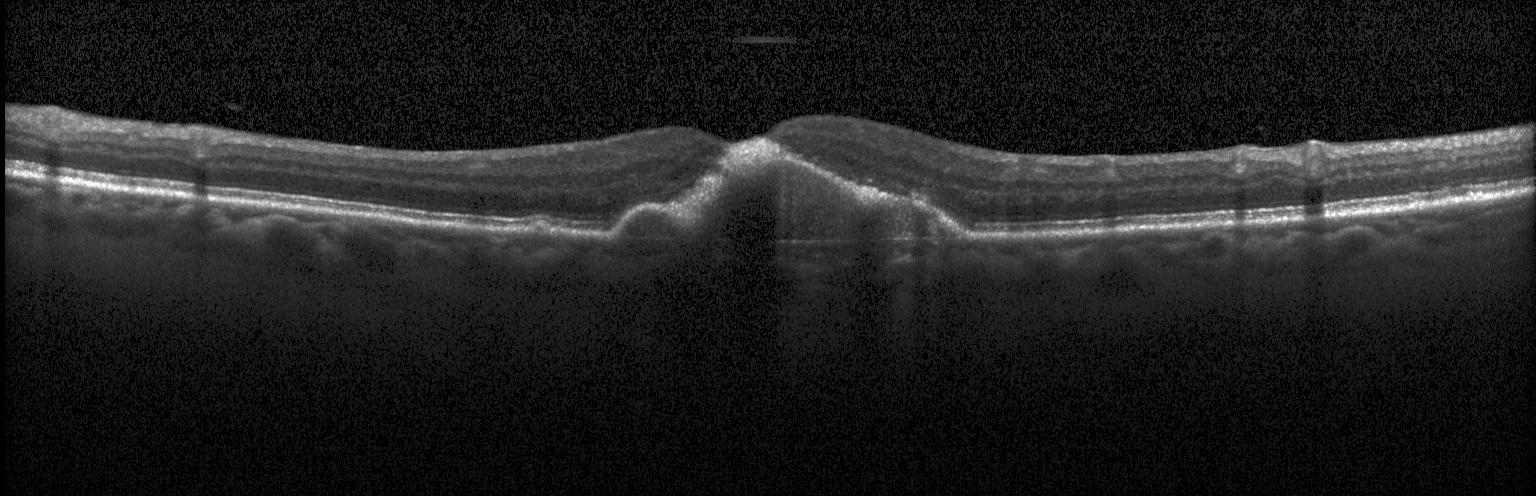 Diagnosis: choroidal neovascularization.